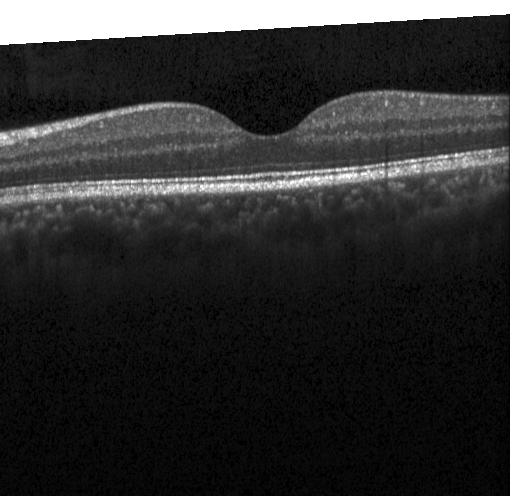 Diagnosis: no CNV, DME, or drusen.